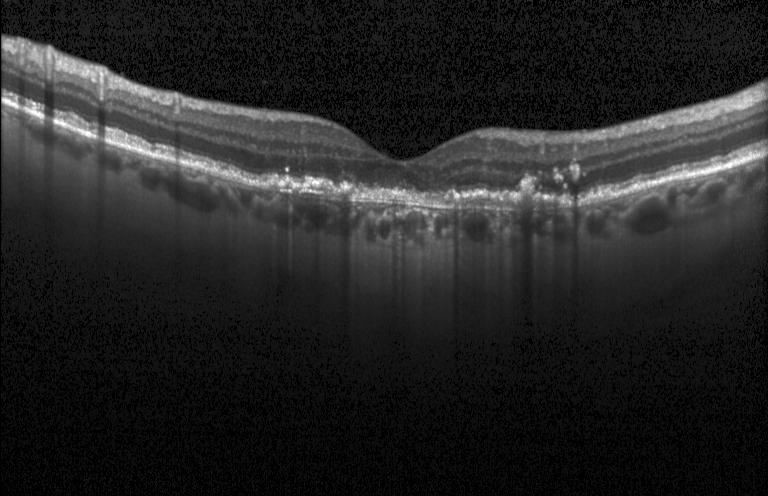
Optical coherence tomography B-scan; spectral-domain OCT; acquired on a Heidelberg Spectralis
Assessment: choroidal neovascularization (CNV).